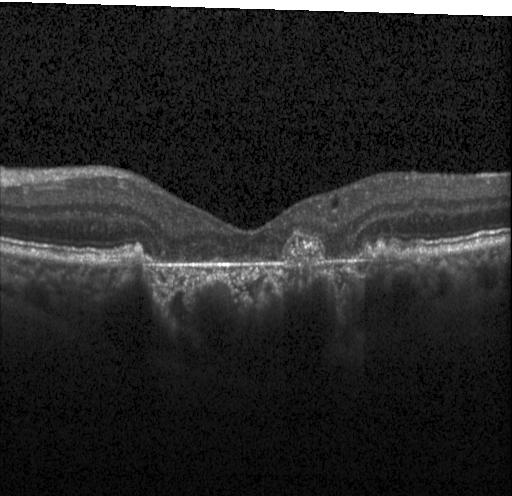
This B-scan demonstrates CNV.